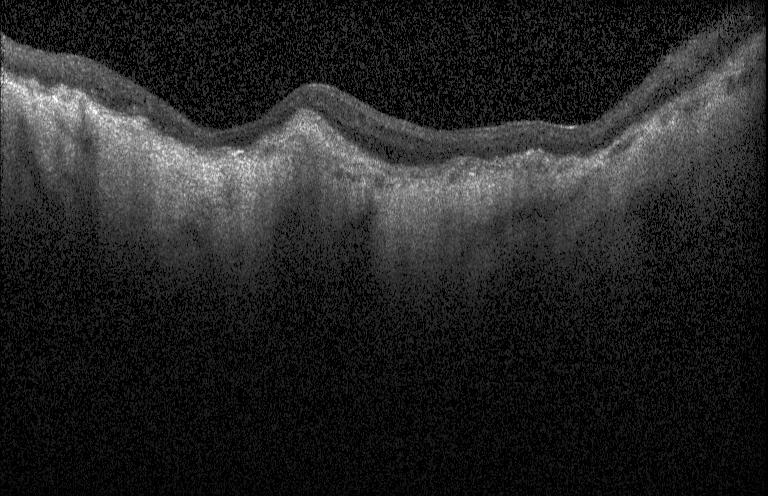

Heidelberg Spectralis OCT system · SD-OCT · centered on the fovea · OCT B-scan
OCT finding: choroidal neovascularization (CNV).